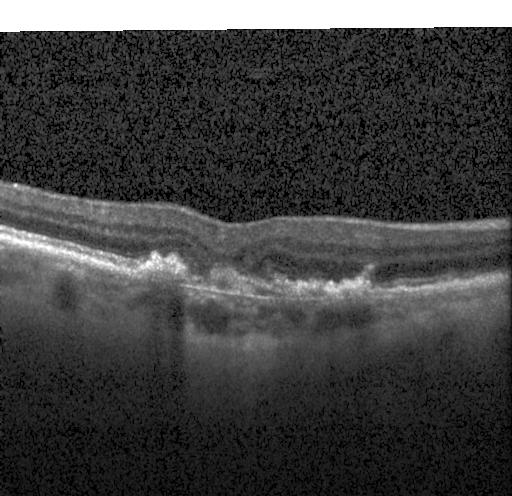
Optical coherence tomography B-scan · instrument: Heidelberg Spectralis.
The scan shows choroidal neovascularization.